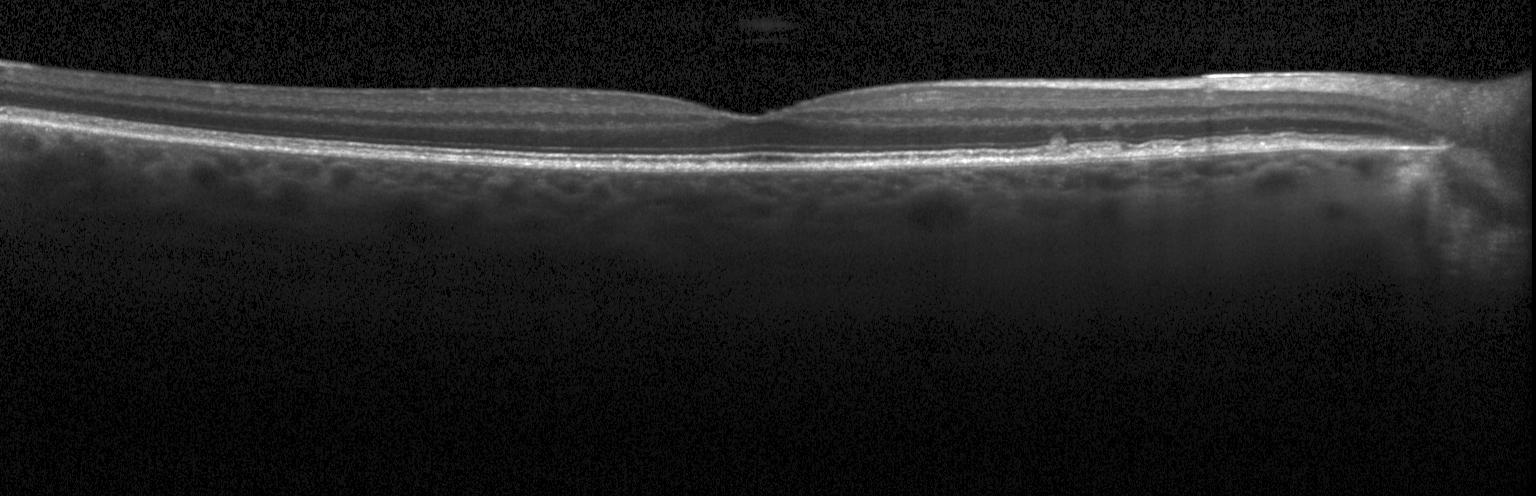 Retinal OCT cross-section. This B-scan demonstrates sub-RPE drusenoid deposits.